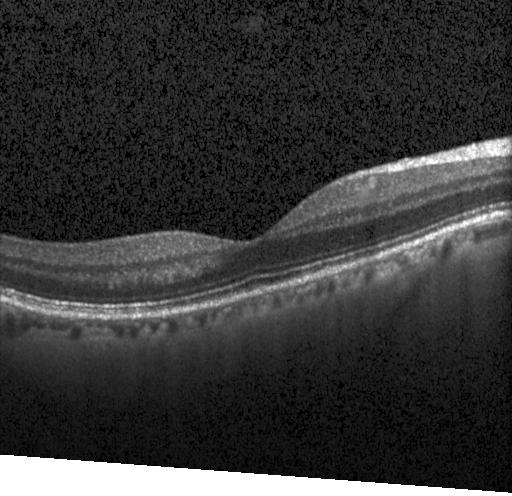

Optical coherence tomography B-scan.
Finding: no choroidal neovascularization, diabetic macular edema, or drusen.